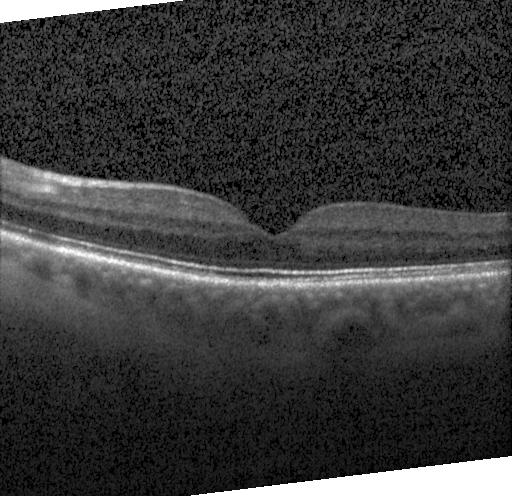

Through the macula, Heidelberg Spectralis, retinal OCT cross-section. Diagnosis: neither choroidal neovascularization, diabetic macular edema, nor drusen.